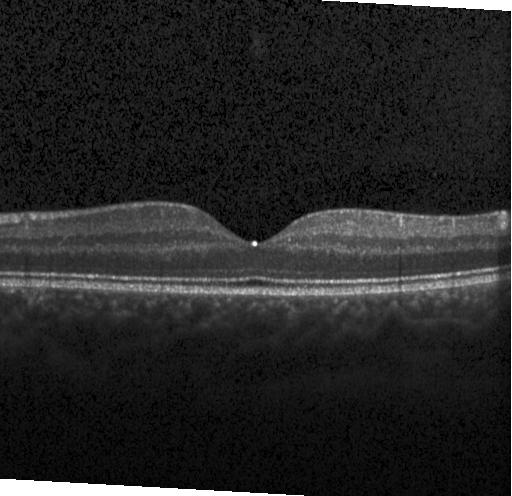
Finding: no choroidal neovascularization, diabetic macular edema, or drusen.